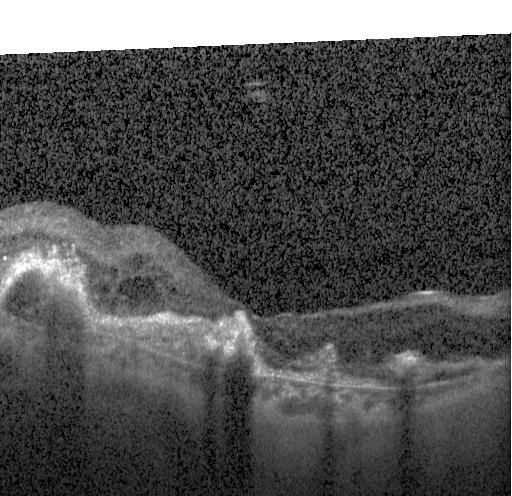

Finding: a choroidal neovascular membrane.